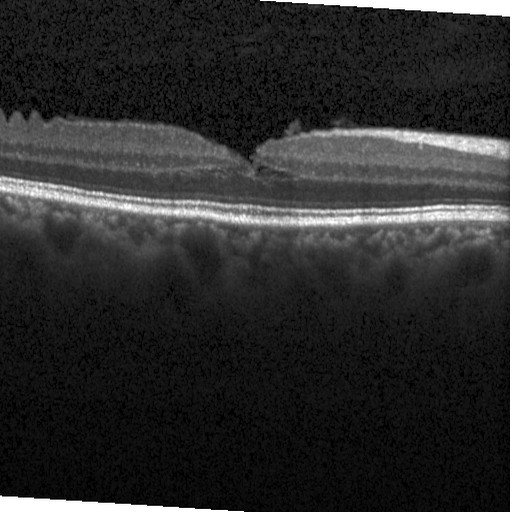
Instrument: Heidelberg Spectralis. Spectral-domain OCT. Retinal OCT cross-section
Assessment: diabetic macular edema (DME).